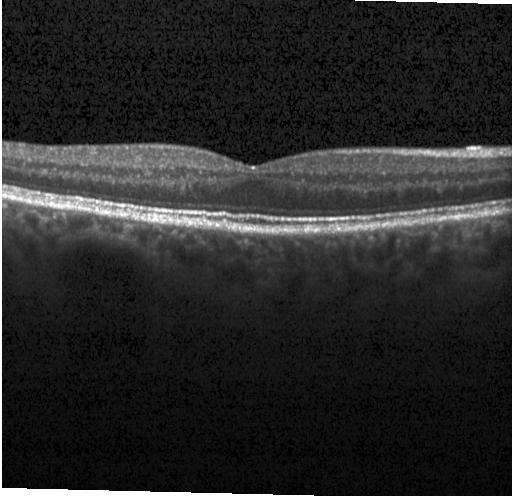
Fovea-centered; optical coherence tomography scan
Macular OCT: neither choroidal neovascularization, diabetic macular edema, nor drusen.